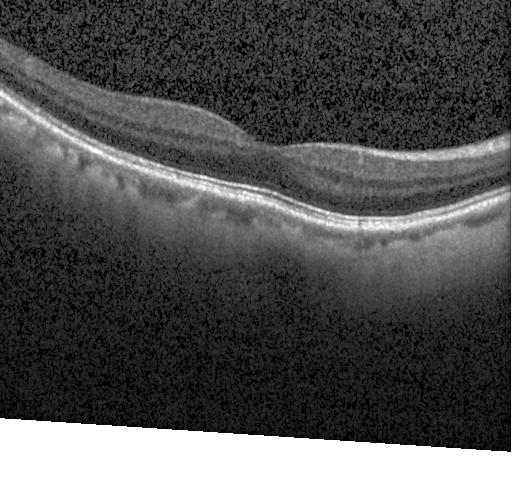
OCT B-scan — The scan shows no choroidal neovascularization, diabetic macular edema, or drusen.